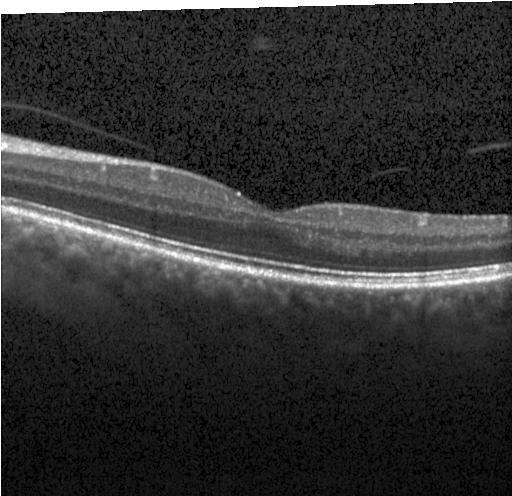
Macular OCT: no choroidal neovascularization, no diabetic macular edema, and no drusen.